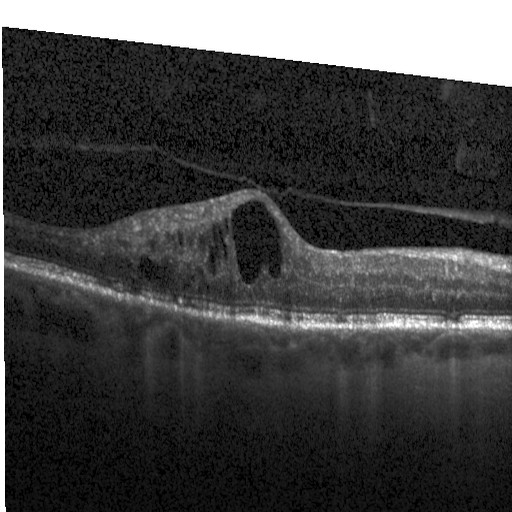 Optical coherence tomography scan
Finding: diabetic macular edema.